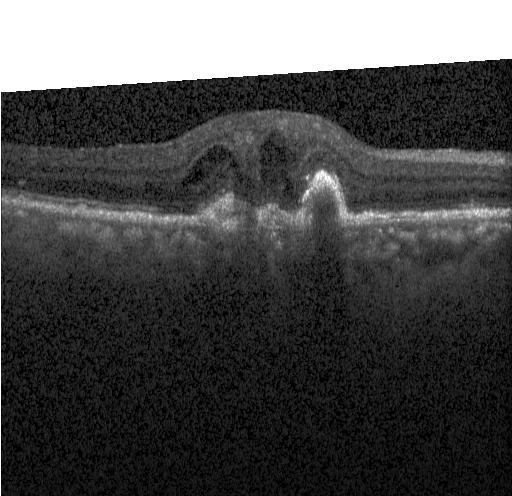 Optical coherence tomography B-scan; horizontal scan through the fovea — Diagnosis: choroidal neovascularization.